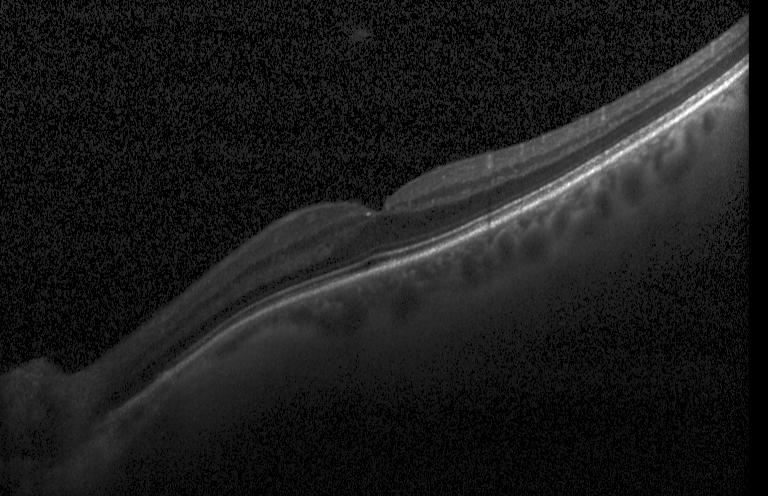

OCT line scan. Acquired on a Heidelberg Spectralis — Diagnosis: no CNV, no DME, and no drusen.